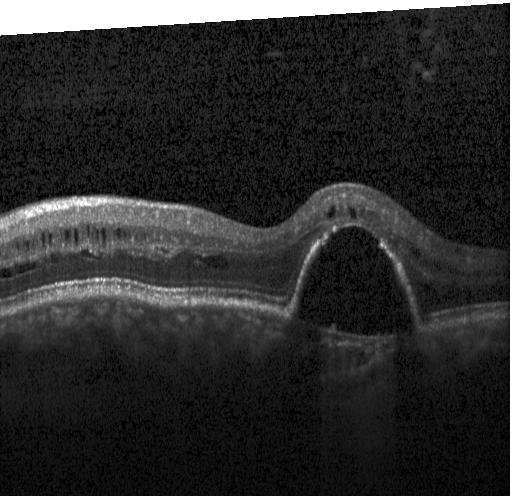

Optical coherence tomography scan. Centered on the fovea. Heidelberg Spectralis OCT system. Spectral-domain optical coherence tomography — A choroidal neovascular membrane.